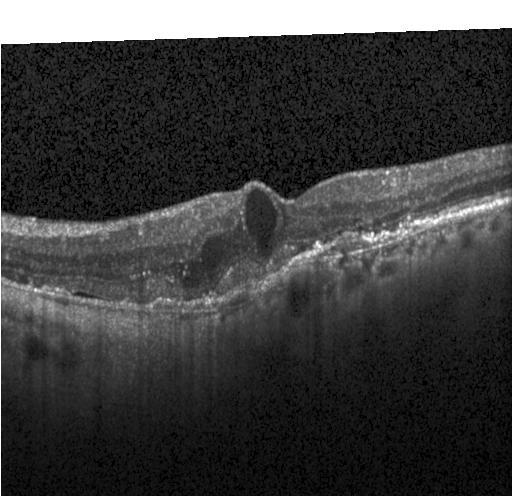
OCT B-scan — The scan shows CNV.